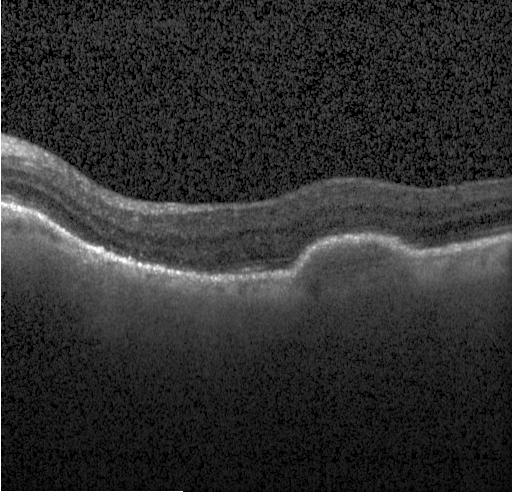

Diagnosis: a choroidal neovascular membrane.